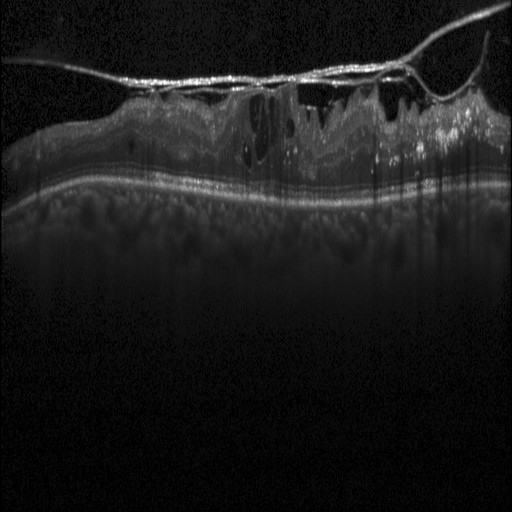 Heidelberg Spectralis OCT system. Macular scan. Optical coherence tomography scan.
Finding: diabetic macular edema.